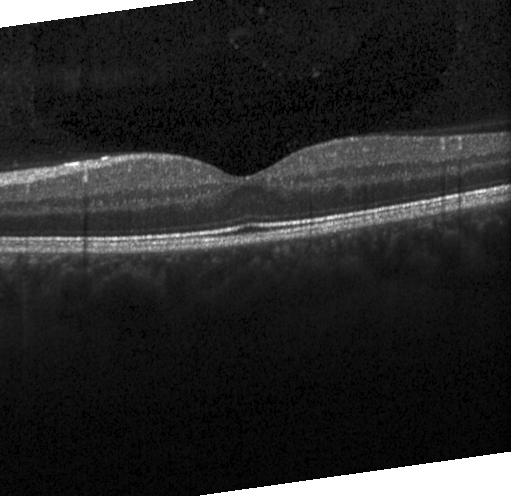
Macular OCT demonstrating neither choroidal neovascularization, diabetic macular edema, nor drusen.